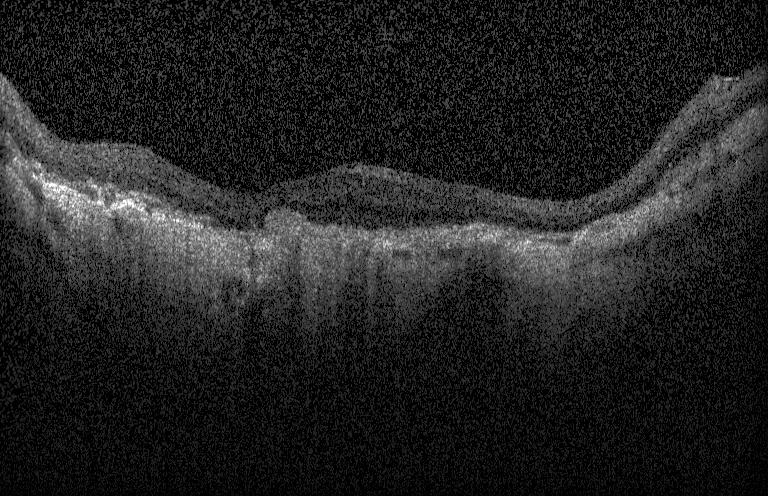

Spectral-domain OCT, instrument: Heidelberg Spectralis, retinal OCT cross-section.
Impression: CNV.